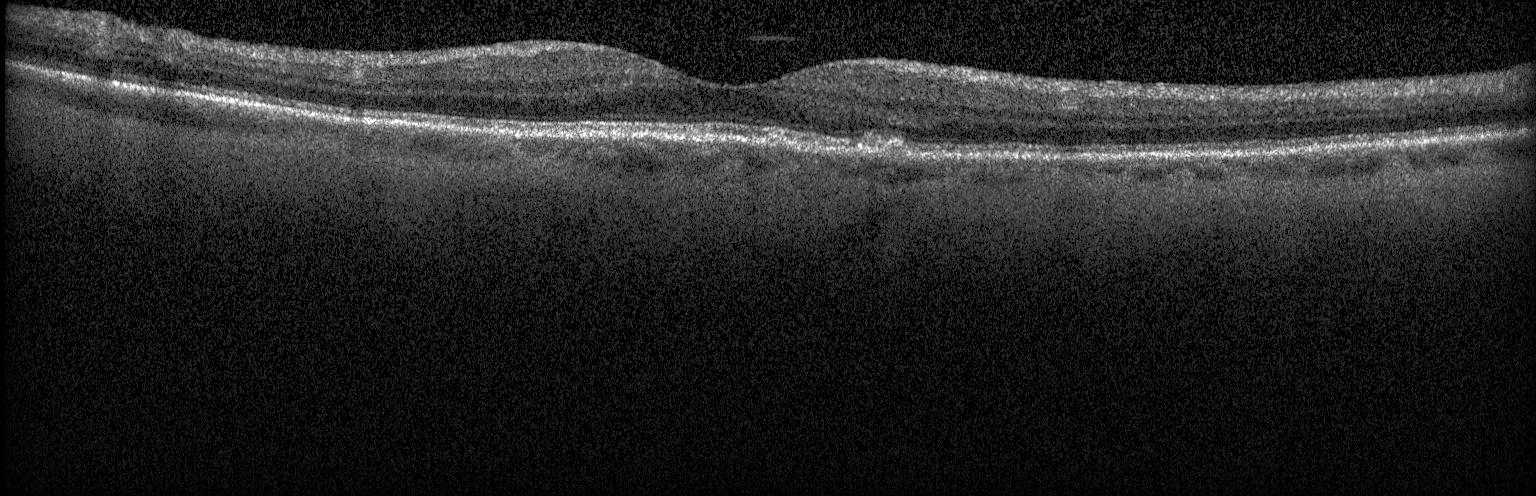 Retinal OCT cross-section · acquired on a Heidelberg Spectralis · horizontal scan through the fovea · spectral-domain OCT.
The scan shows multiple drusen.